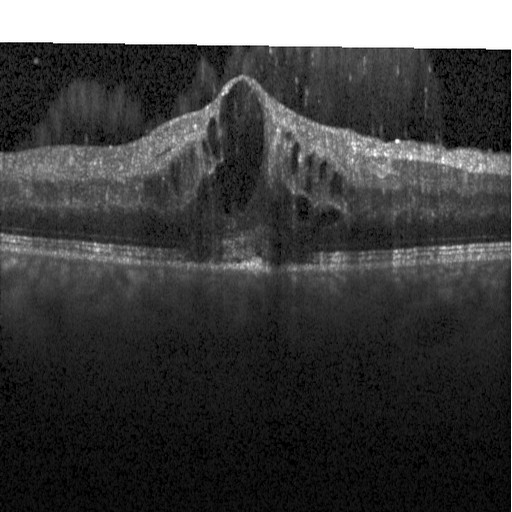 Acquired on a Heidelberg Spectralis; optical coherence tomography B-scan; fovea-centered; SD-OCT. This B-scan demonstrates DME.